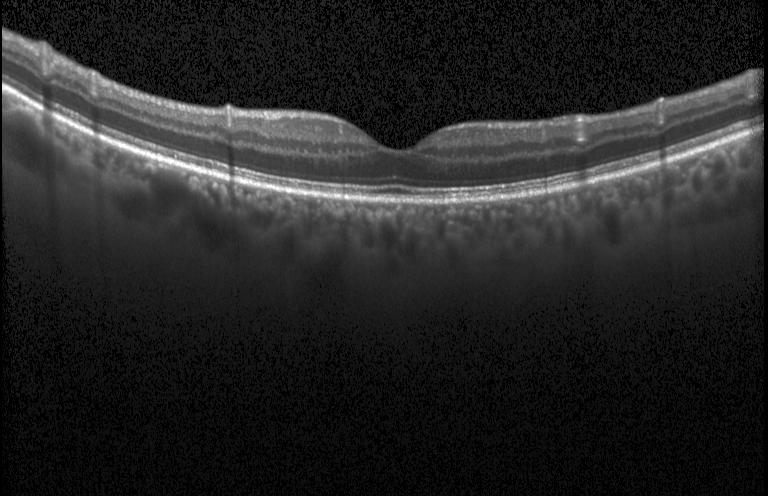 Finding: no CNV, no DME, and no drusen.